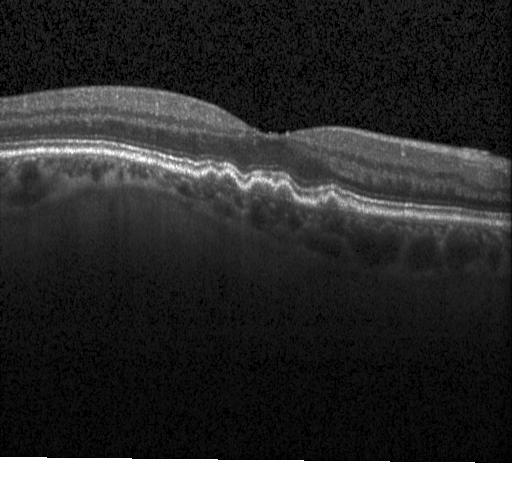
OCT finding: sub-RPE drusenoid deposits.